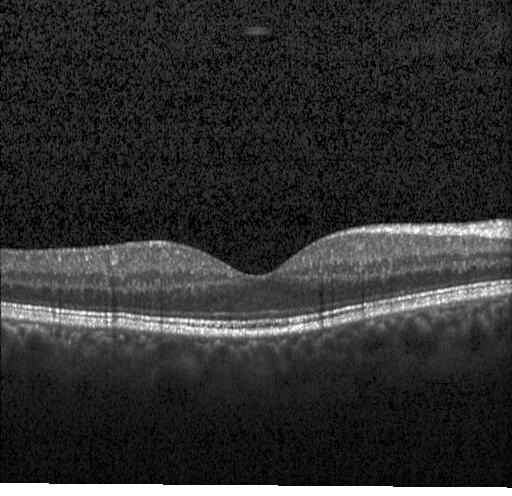 Through the macula, retinal OCT cross-section, spectral-domain optical coherence tomography
Impression: neither choroidal neovascularization, diabetic macular edema, nor drusen.